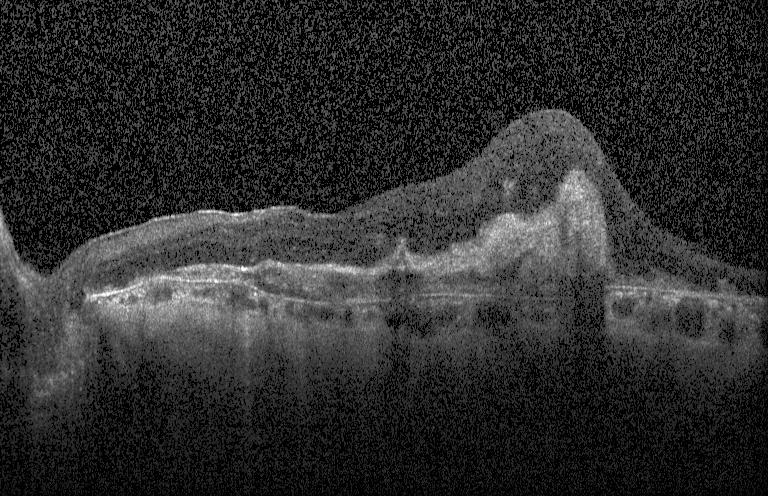
Retinal OCT cross-section showing CNV.